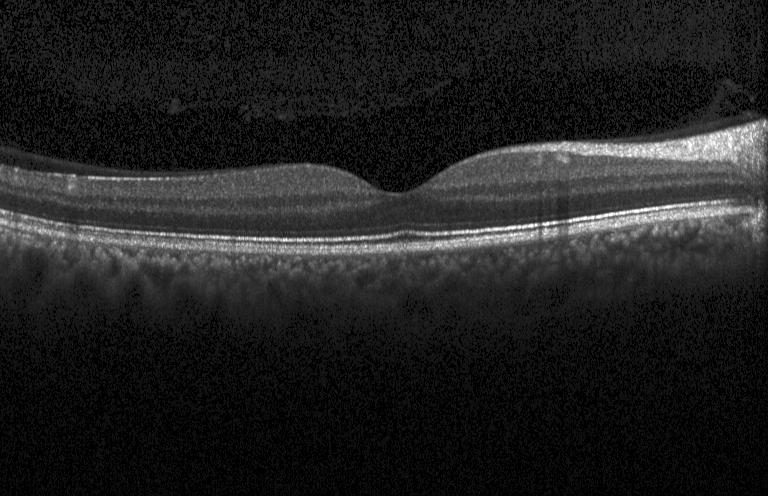
Heidelberg Spectralis. Through the macula. SD-OCT. Retinal OCT cross-section. Macular OCT: no evidence of choroidal neovascularization, diabetic macular edema, or drusen.